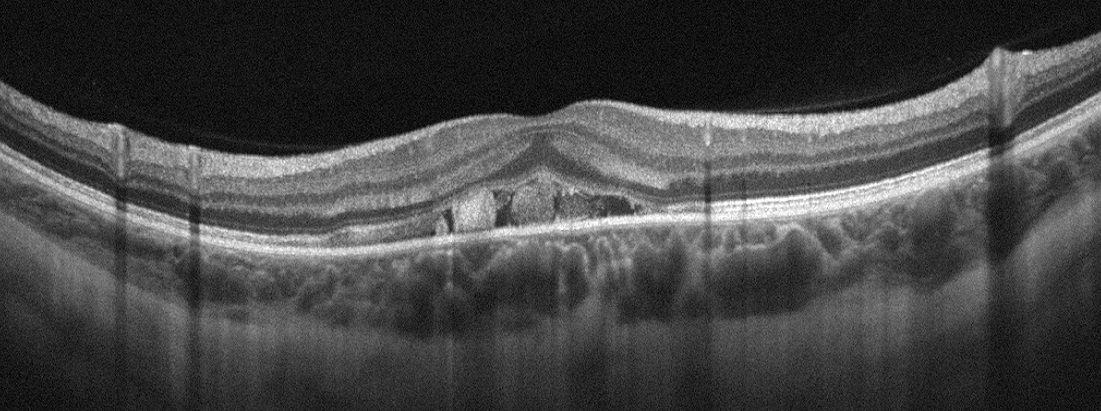

Diagnosis: age-related macular degeneration (AMD).